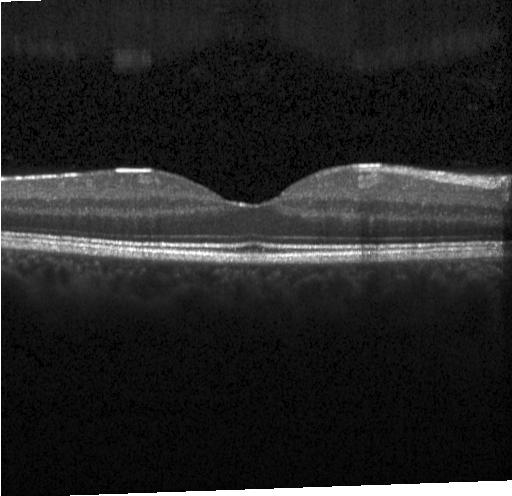
Spectral-domain OCT · optical coherence tomography scan.
Macular OCT: neither choroidal neovascularization, diabetic macular edema, nor drusen.